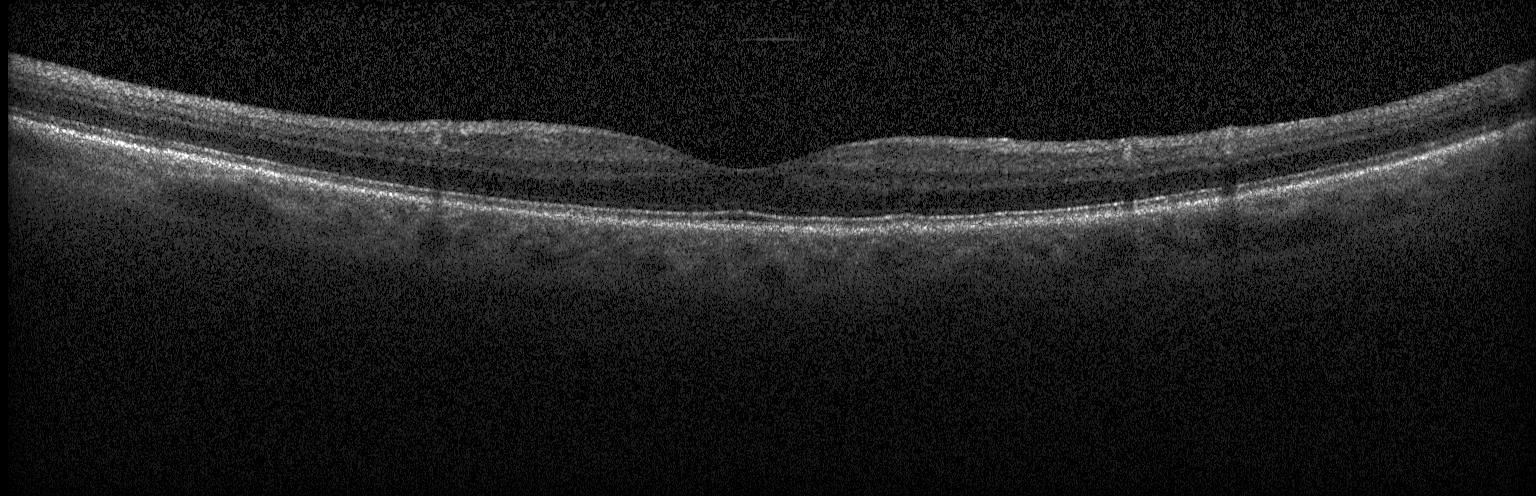

SD-OCT, OCT line scan.
Impression: no CNV, no DME, and no drusen.